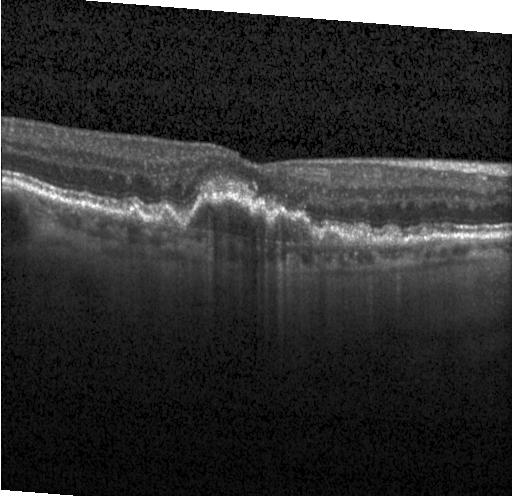
Macular OCT demonstrating a choroidal neovascular membrane.